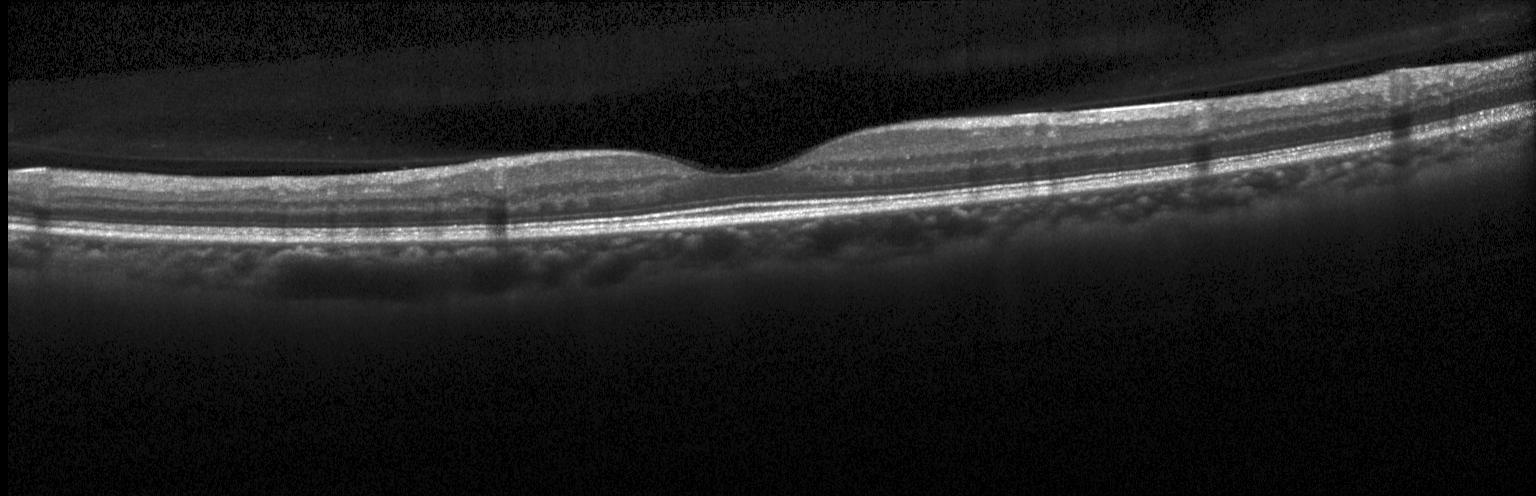
Heidelberg Spectralis, horizontal scan through the fovea, retinal OCT B-scan. Diagnosis: no CNV, no DME, and no drusen.